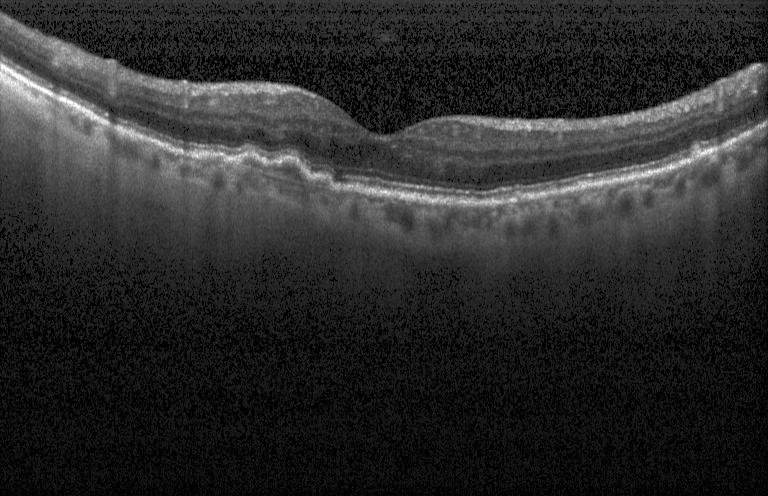
Diagnosis: sub-RPE drusenoid deposits.